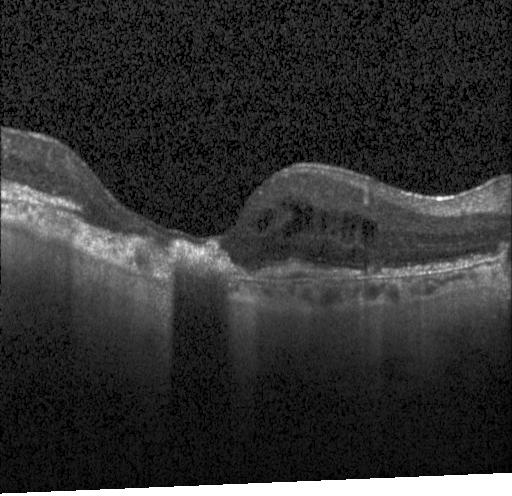

Diagnosis: choroidal neovascularization.